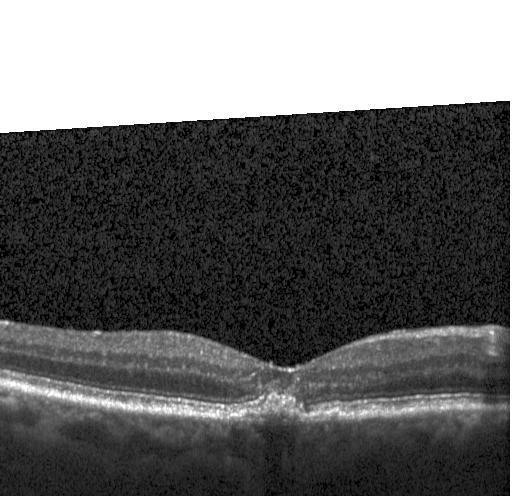 Instrument: Heidelberg Spectralis, retinal OCT B-scan, spectral-domain OCT
This B-scan demonstrates multiple drusen.